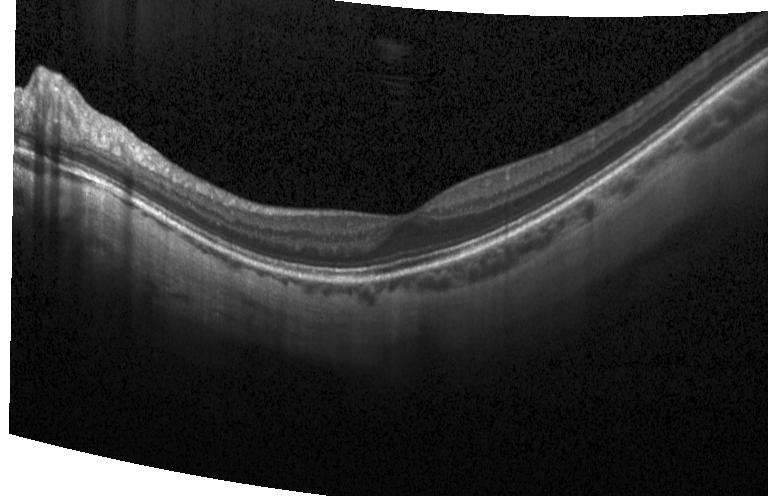 The scan shows no choroidal neovascularization, diabetic macular edema, or drusen.